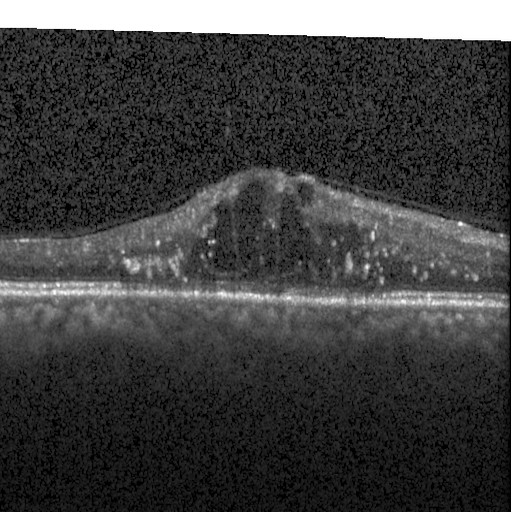

Finding: diabetic macular edema.